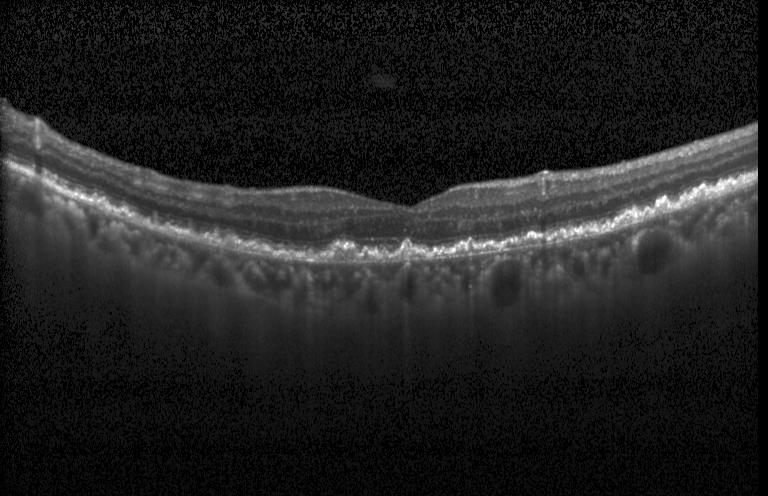 Optical coherence tomography B-scan.
Multiple drusen.